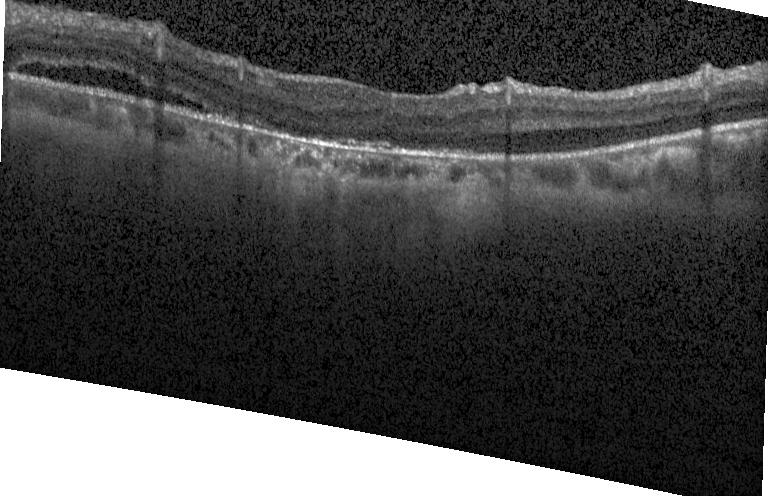
Retinal OCT B-scan, through the macula, acquired on a Heidelberg Spectralis. Diagnosis: a choroidal neovascular membrane.